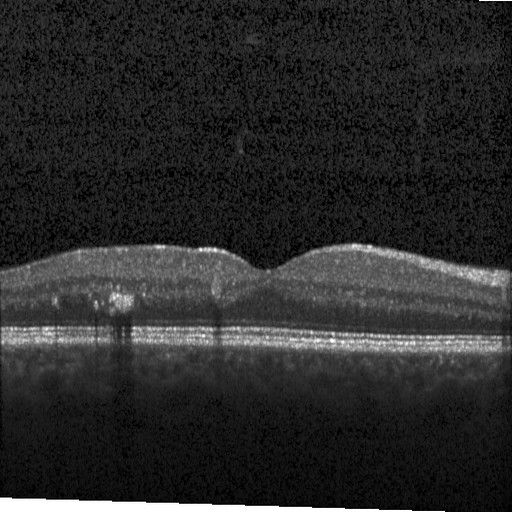

Optical coherence tomography B-scan; through the macula; spectral-domain OCT
This B-scan demonstrates diabetic macular edema (DME).